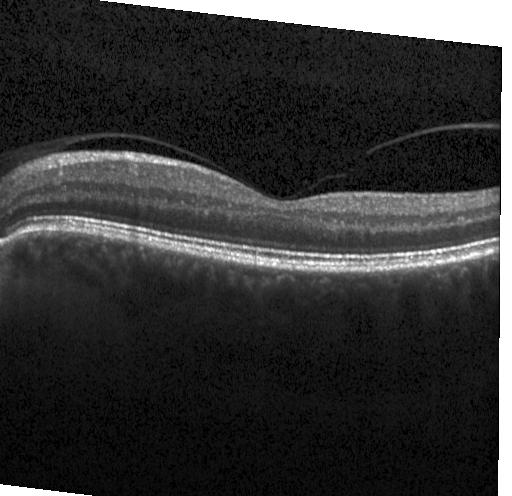 Instrument: Heidelberg Spectralis; retinal OCT B-scan; SD-OCT.
Diagnosis: no evidence of choroidal neovascularization, diabetic macular edema, or drusen.